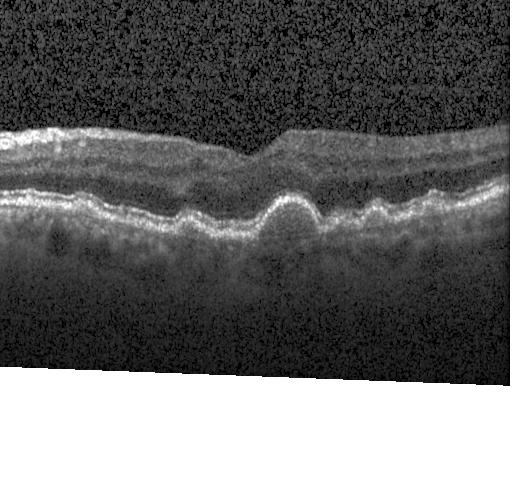 Macular OCT demonstrating multiple drusen.